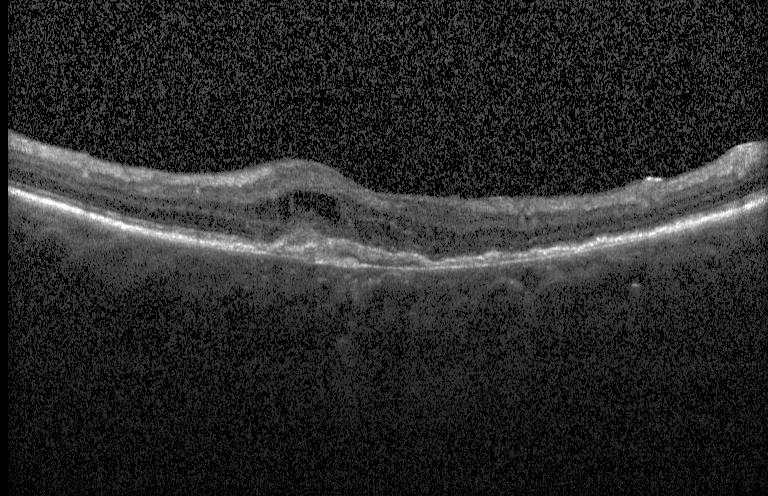

Dx: choroidal neovascularization (CNV).